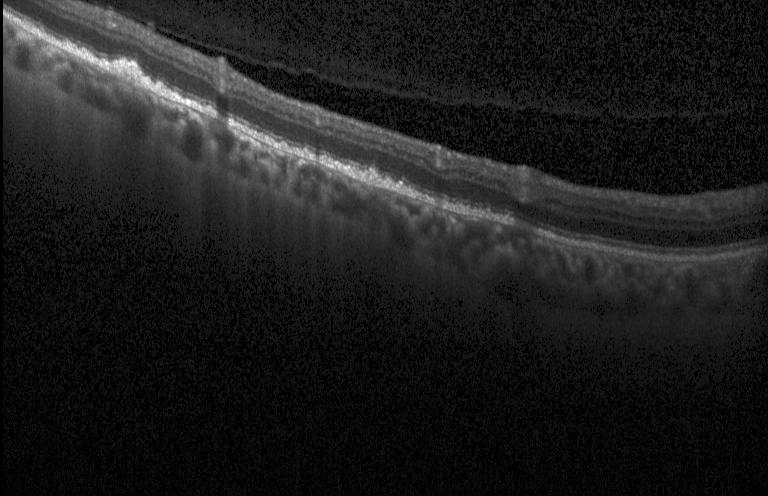

Finding: multiple drusen.